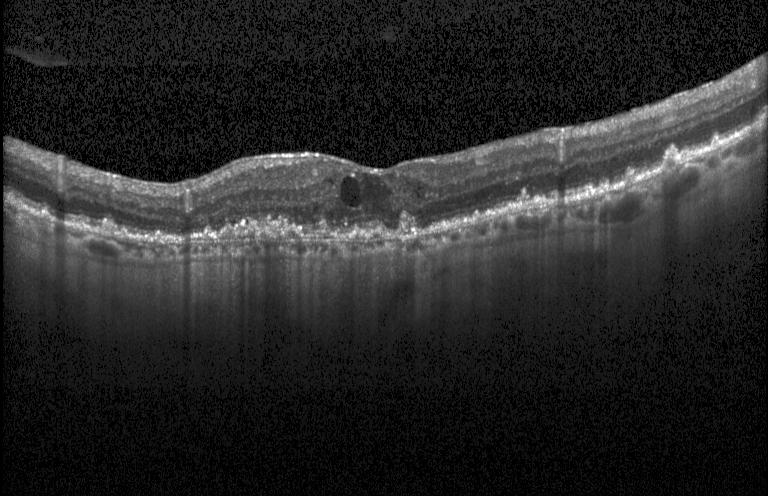 Through the macula. Spectral-domain OCT. OCT line scan
Diagnosis: choroidal neovascularization.